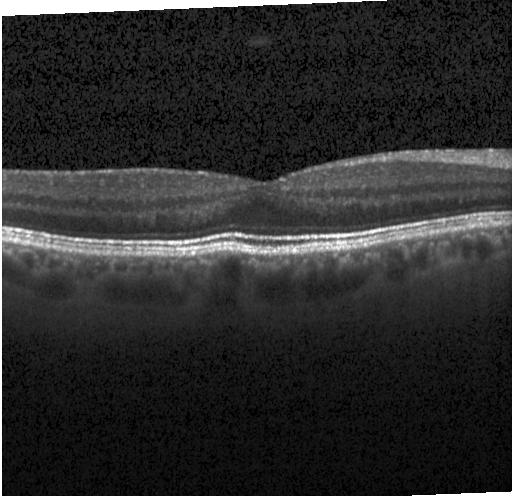

Optical coherence tomography B-scan.
Macular OCT: no choroidal neovascularization, diabetic macular edema, or drusen.